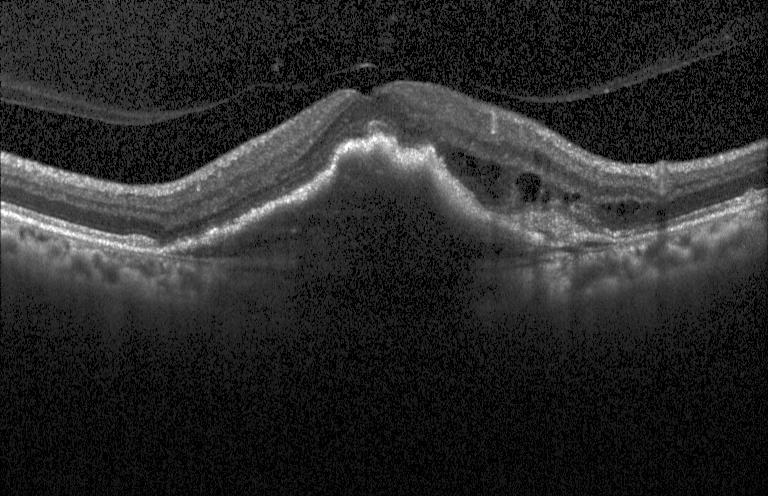
A choroidal neovascular membrane.